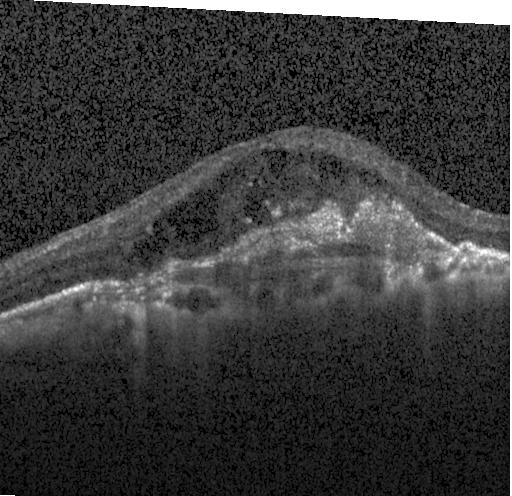

Spectral-domain OCT B-scan: choroidal neovascularization (CNV).